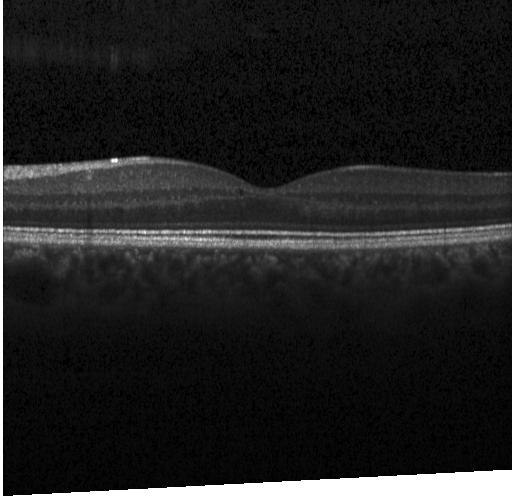 Assessment: no CNV, DME, or drusen.